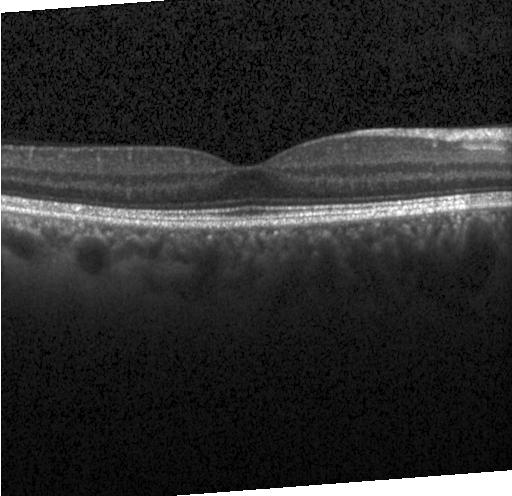 Impression: no CNV, DME, or drusen.